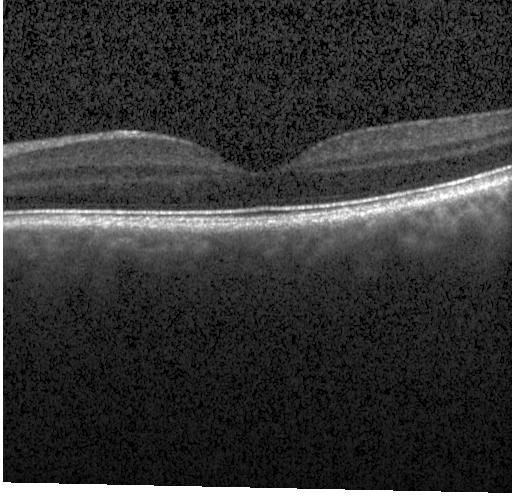
OCT B-scan — Finding: no CNV, DME, or drusen.